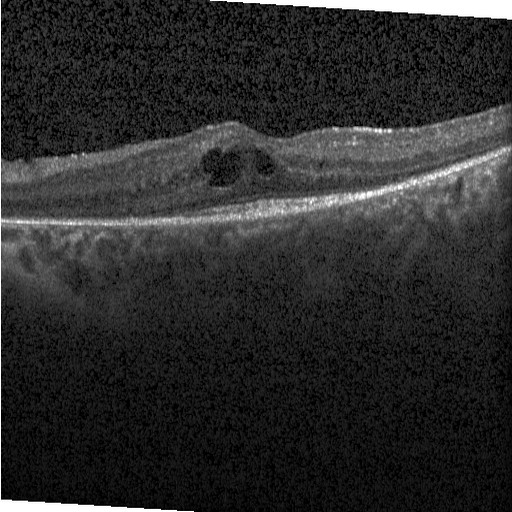

Fovea-centered. Retinal OCT cross-section. Spectral-domain optical coherence tomography
OCT finding: diabetic macular edema (DME).